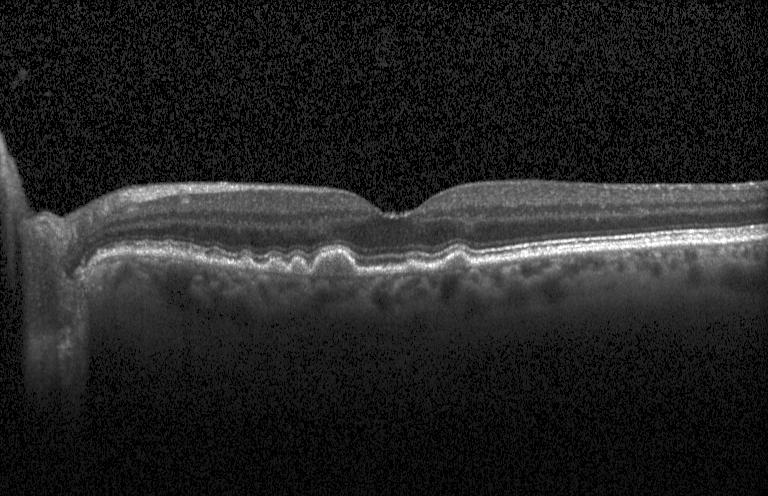
Assessment: multiple drusen.